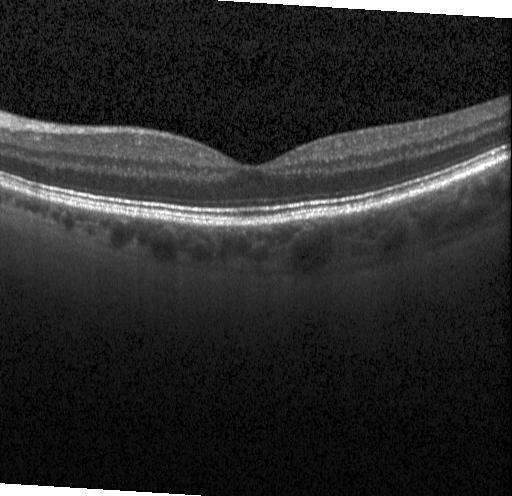

Heidelberg Spectralis OCT system, optical coherence tomography scan. Diagnosis: no choroidal neovascularization, diabetic macular edema, or drusen.